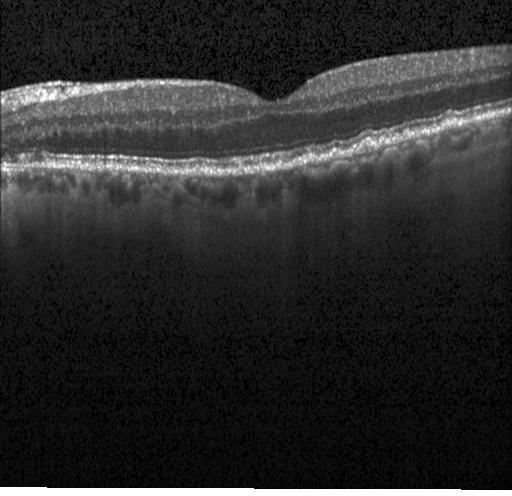
Retinal OCT B-scan, SD-OCT, acquired on a Heidelberg Spectralis.
Assessment: multiple drusen.